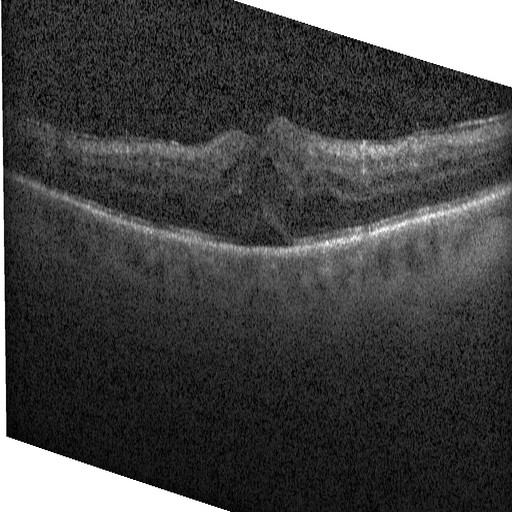

Acquired on a Heidelberg Spectralis. OCT B-scan. SD-OCT. Macular scan — Impression: diabetic macular edema (DME).